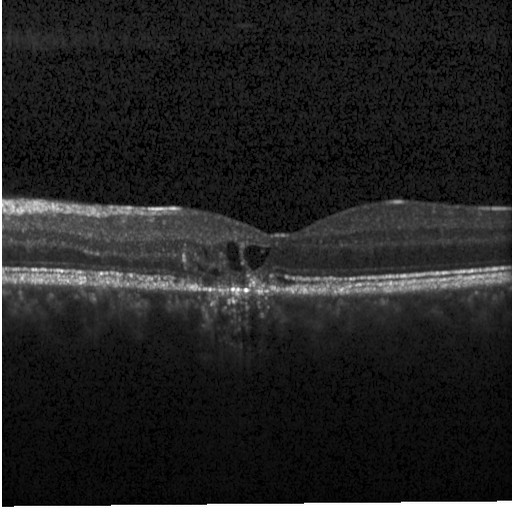 OCT line scan
Macular OCT: diabetic macular edema (DME).